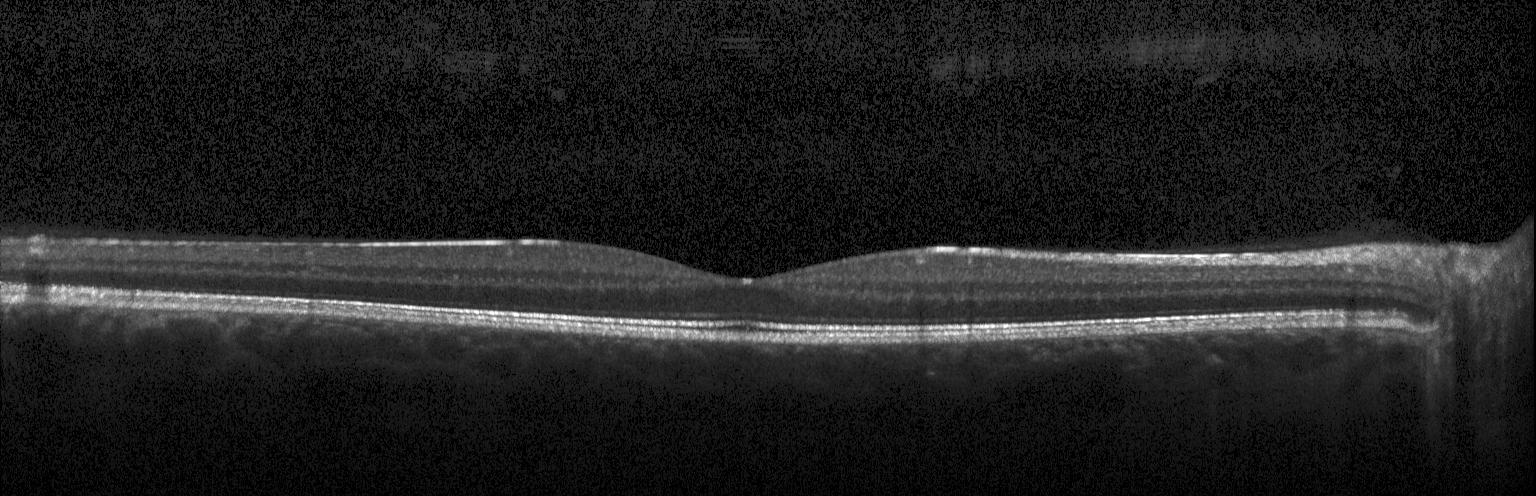 Impression: no choroidal neovascularization, no diabetic macular edema, and no drusen.